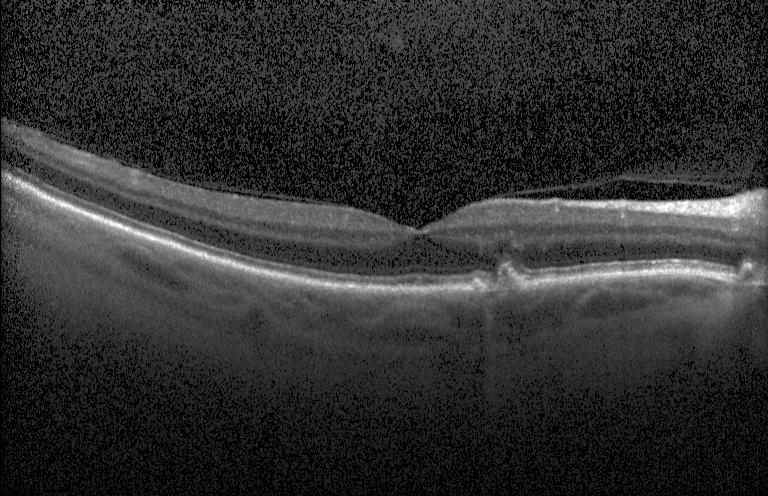 Horizontal scan through the fovea · retinal OCT cross-section · spectral-domain optical coherence tomography · Heidelberg Spectralis. Assessment: drusen.